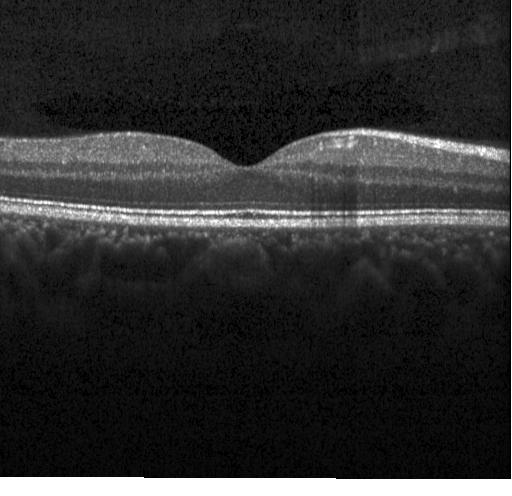
Retinal OCT cross-section · Heidelberg Spectralis OCT system · spectral-domain OCT — Assessment: no CNV, DME, or drusen.